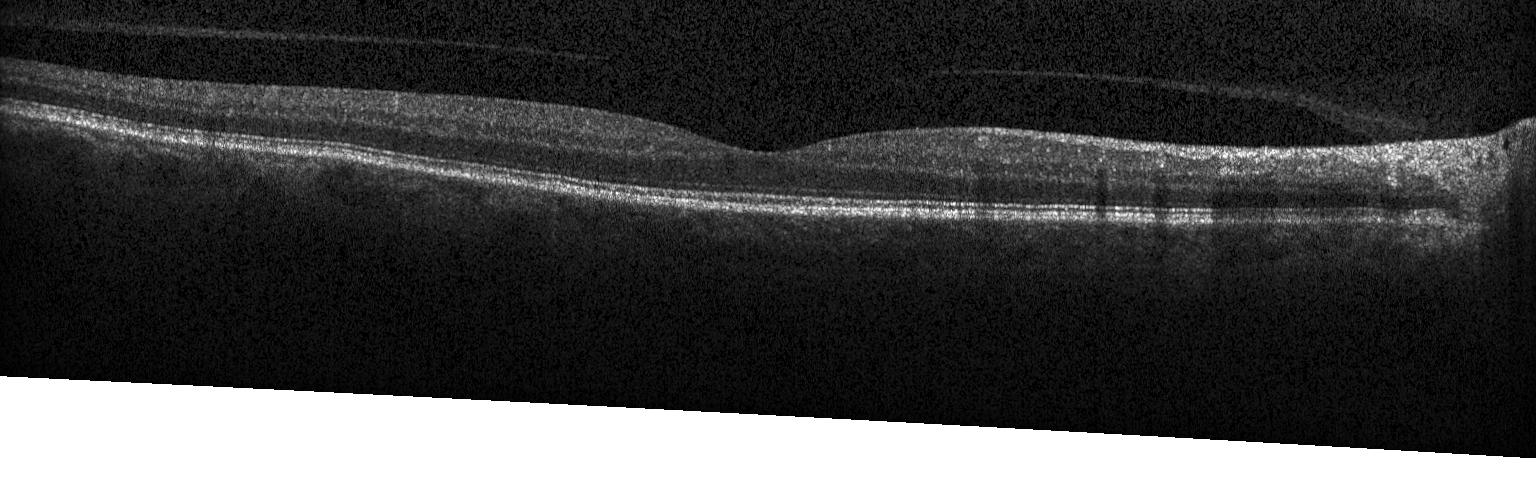 Optical coherence tomography scan. No choroidal neovascularization, diabetic macular edema, or drusen.